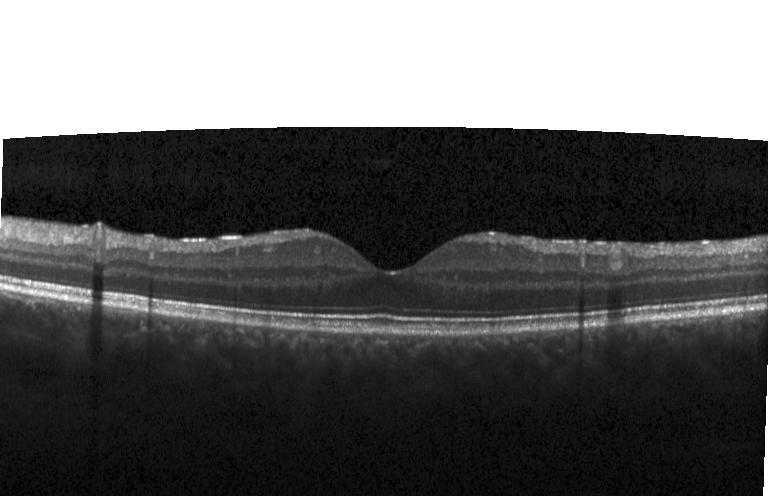

Spectral-domain OCT. Retinal OCT B-scan. Instrument: Heidelberg Spectralis. Centered on the fovea
OCT finding: no choroidal neovascularization, no diabetic macular edema, and no drusen.